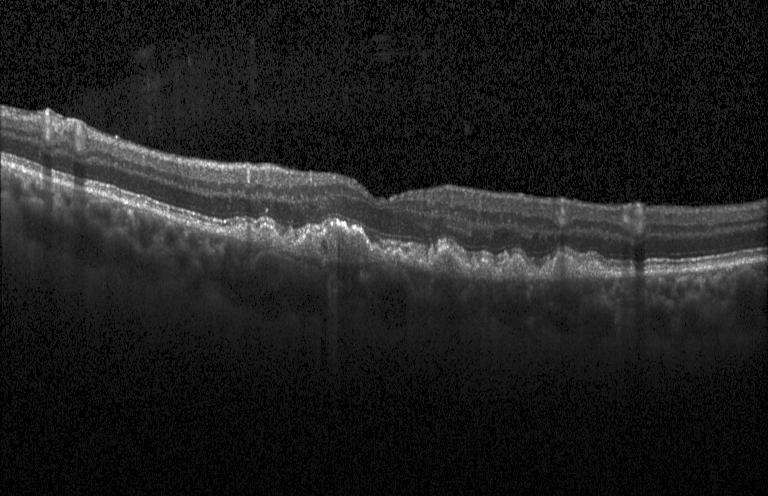
Instrument: Heidelberg Spectralis. Retinal OCT cross-section. The scan shows a choroidal neovascular membrane.